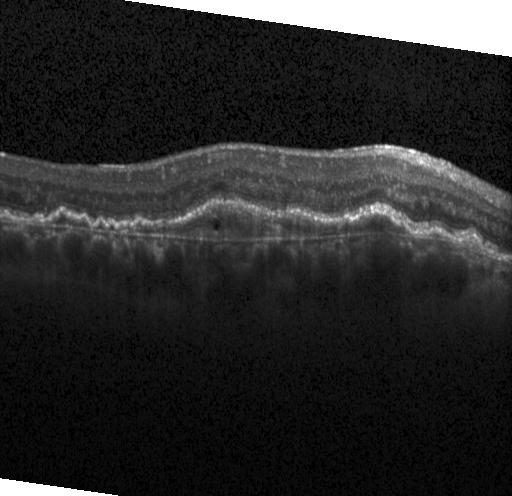

The scan shows choroidal neovascularization.